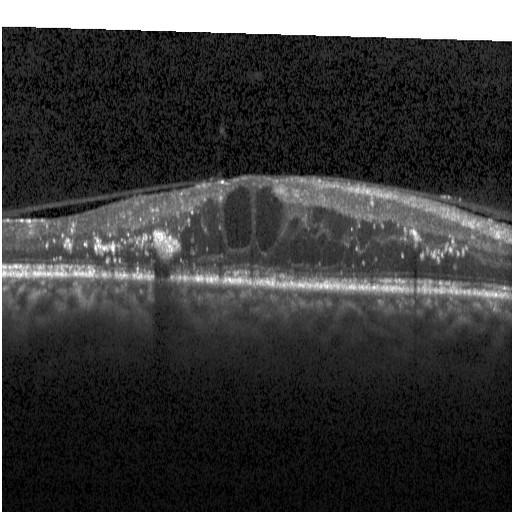
SD-OCT, through the macula, retinal OCT cross-section. Finding: diabetic macular edema.